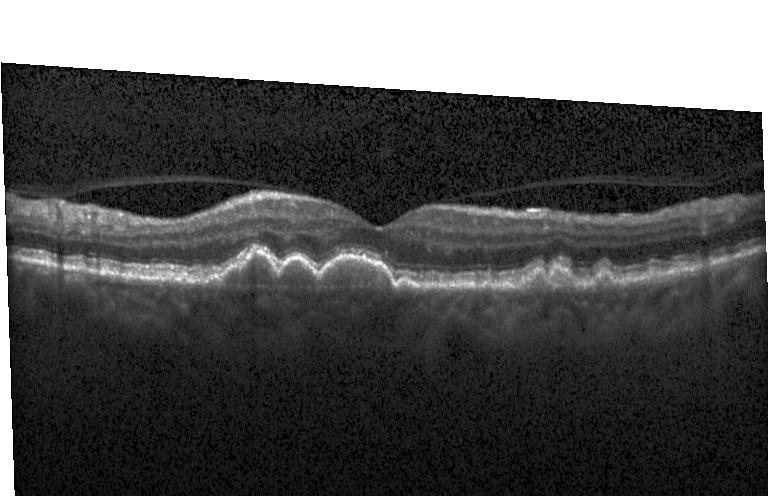 Spectral-domain optical coherence tomography. Optical coherence tomography scan.
Impression: sub-RPE drusenoid deposits.